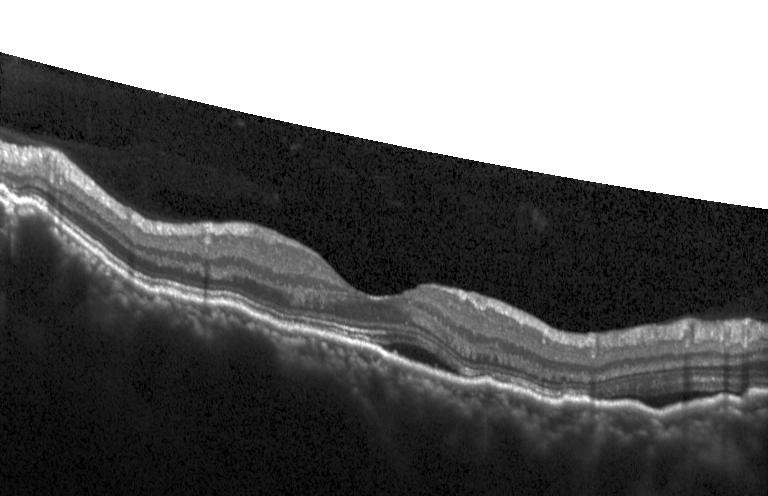

OCT line scan. Choroidal neovascularization (CNV).